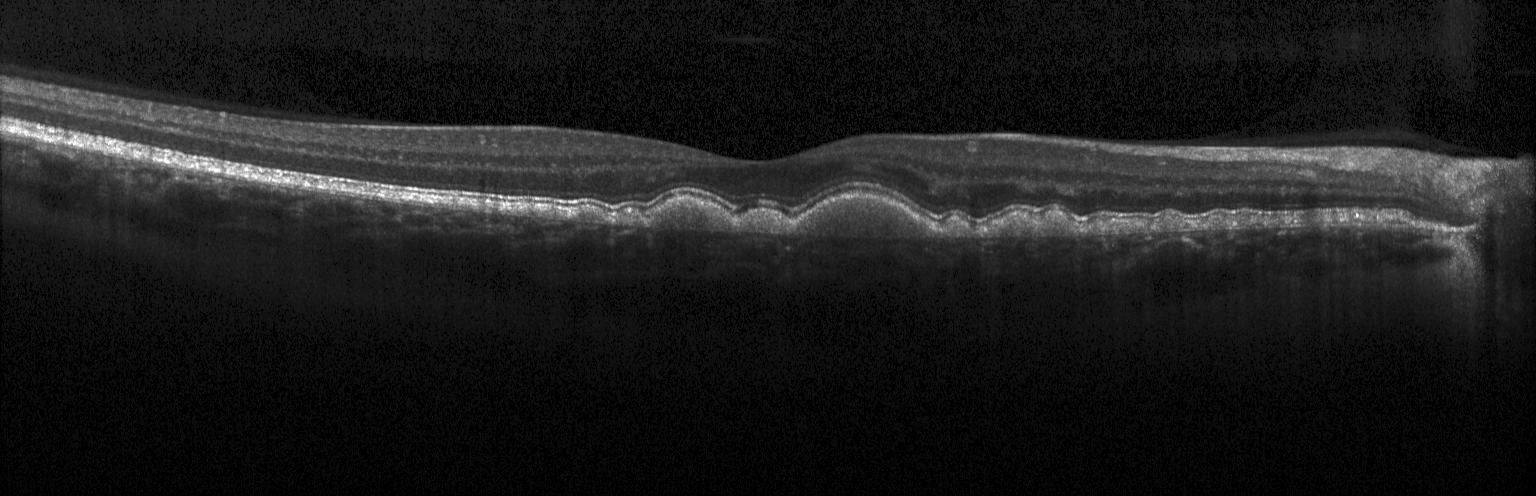
Acquired on a Heidelberg Spectralis, macular scan, OCT B-scan. Finding: sub-RPE drusenoid deposits.